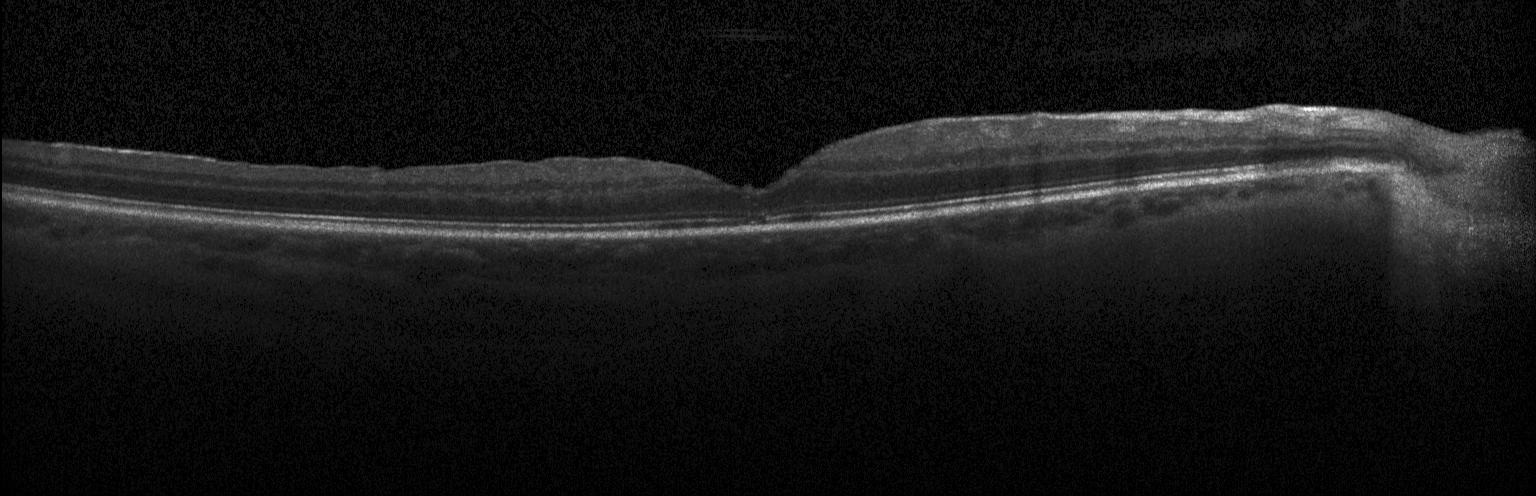 This B-scan demonstrates no evidence of CNV, DME, or drusen.